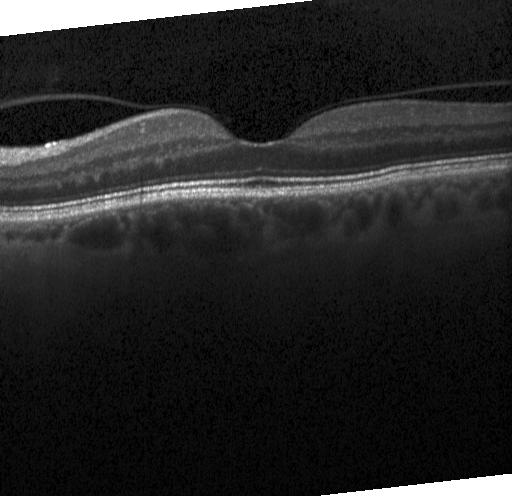
Optical coherence tomography B-scan; centered on the fovea; Heidelberg Spectralis OCT system — Dx: neither choroidal neovascularization, diabetic macular edema, nor drusen.